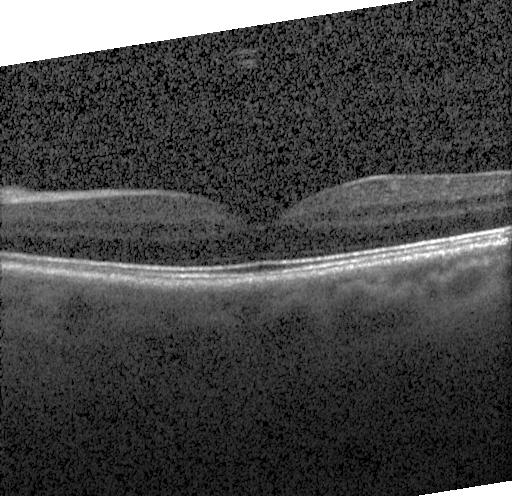
The scan shows no choroidal neovascularization, diabetic macular edema, or drusen.